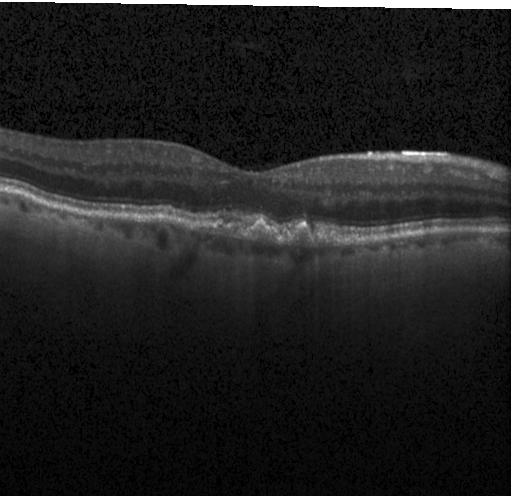
Through the macula; optical coherence tomography scan; SD-OCT. This B-scan demonstrates drusen.